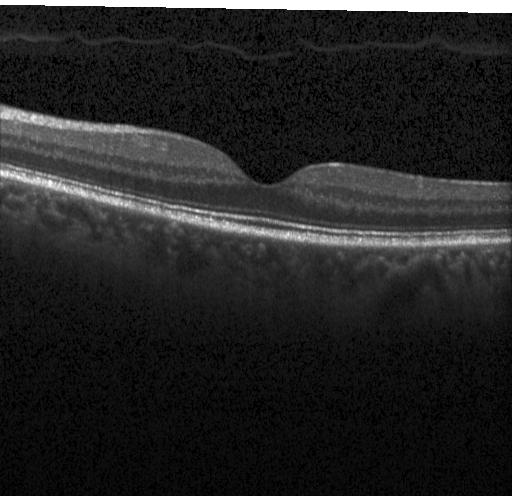
Retinal OCT B-scan; through the macula; instrument: Heidelberg Spectralis; spectral-domain optical coherence tomography.
Finding: no evidence of choroidal neovascularization, diabetic macular edema, or drusen.